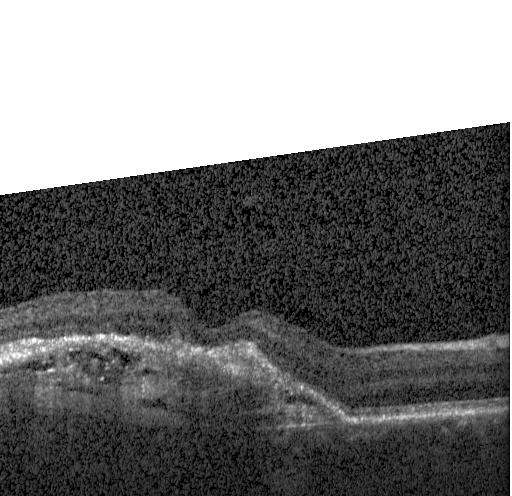

Assessment: a choroidal neovascular membrane.